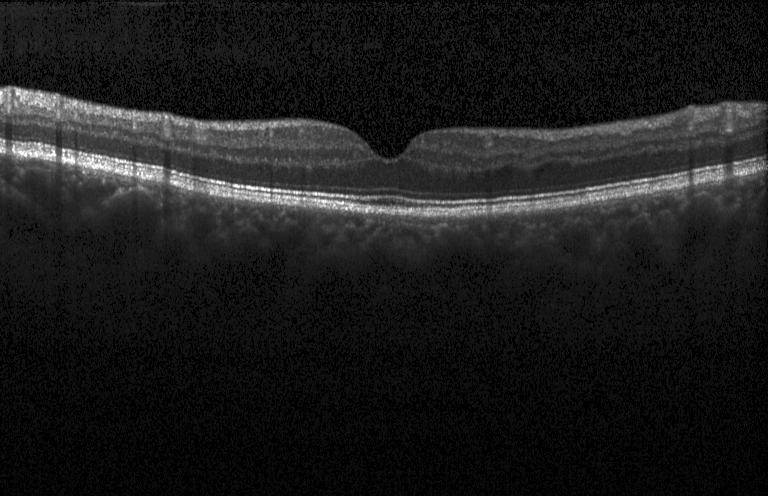
OCT B-scan. Horizontal scan through the fovea. Acquired on a Heidelberg Spectralis. SD-OCT.
The scan shows neither choroidal neovascularization, diabetic macular edema, nor drusen.